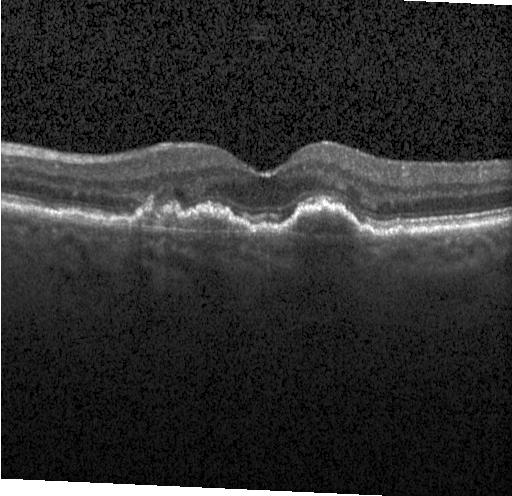

Impression: choroidal neovascularization (CNV).